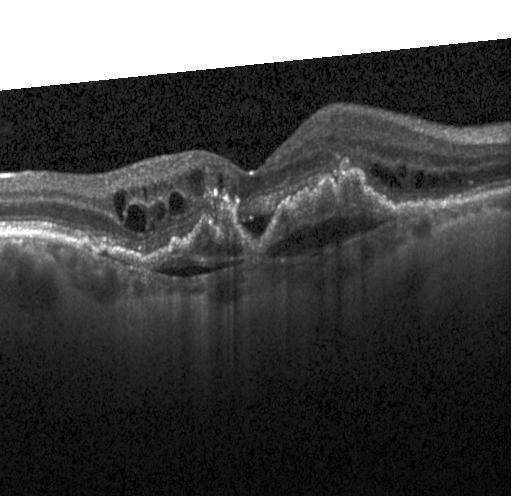 Optical coherence tomography B-scan, through the macula.
Diagnosis: choroidal neovascularization (CNV).